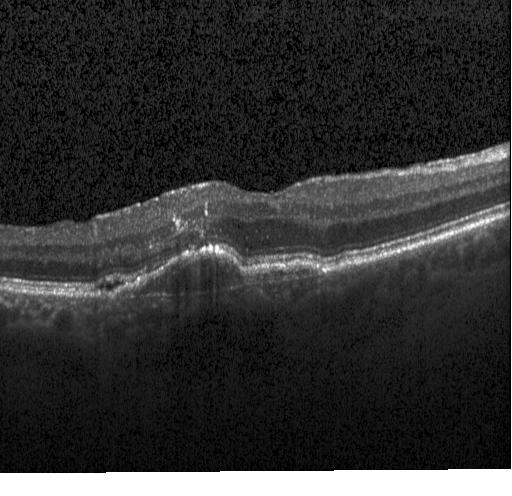

SD-OCT; OCT line scan; Heidelberg Spectralis OCT system; macular scan.
OCT finding: a choroidal neovascular membrane.